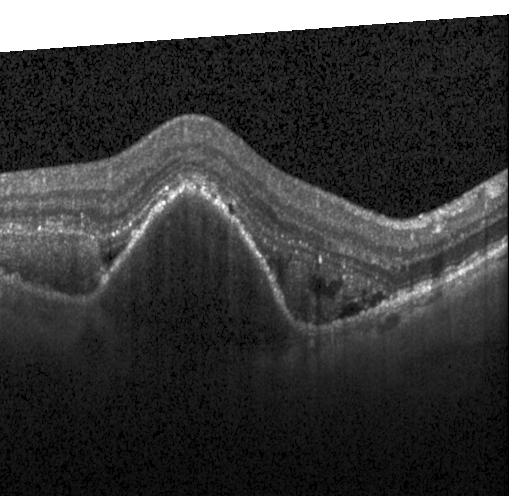

Macular OCT demonstrating choroidal neovascularization.